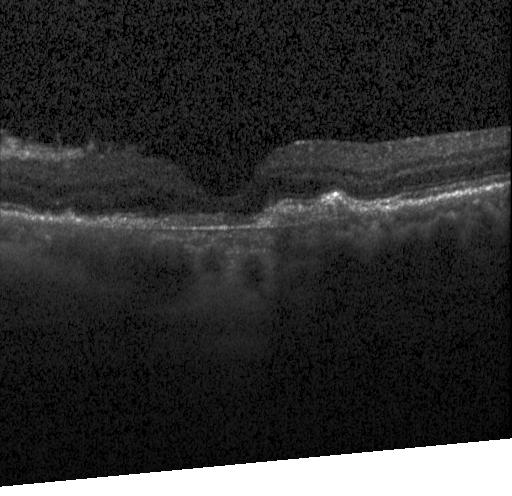 Spectral-domain optical coherence tomography. Heidelberg Spectralis. Retinal OCT B-scan. Fovea-centered. This B-scan demonstrates choroidal neovascularization (CNV).